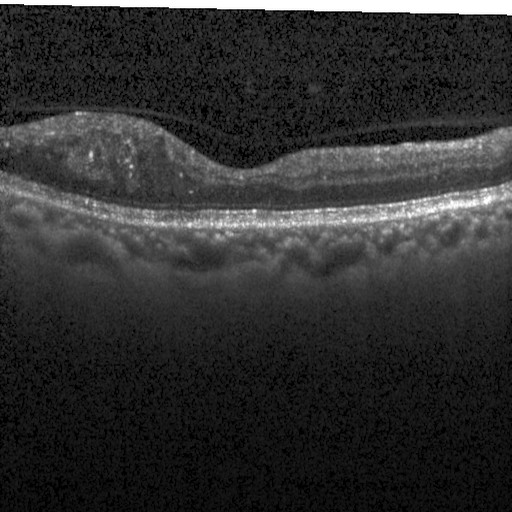 Macular OCT: diabetic macular edema.